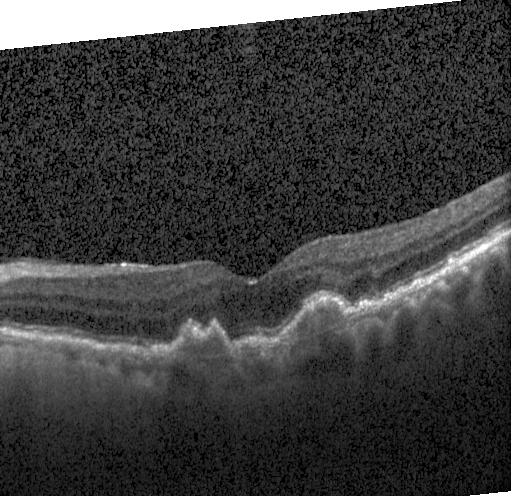 Dx: choroidal neovascularization.